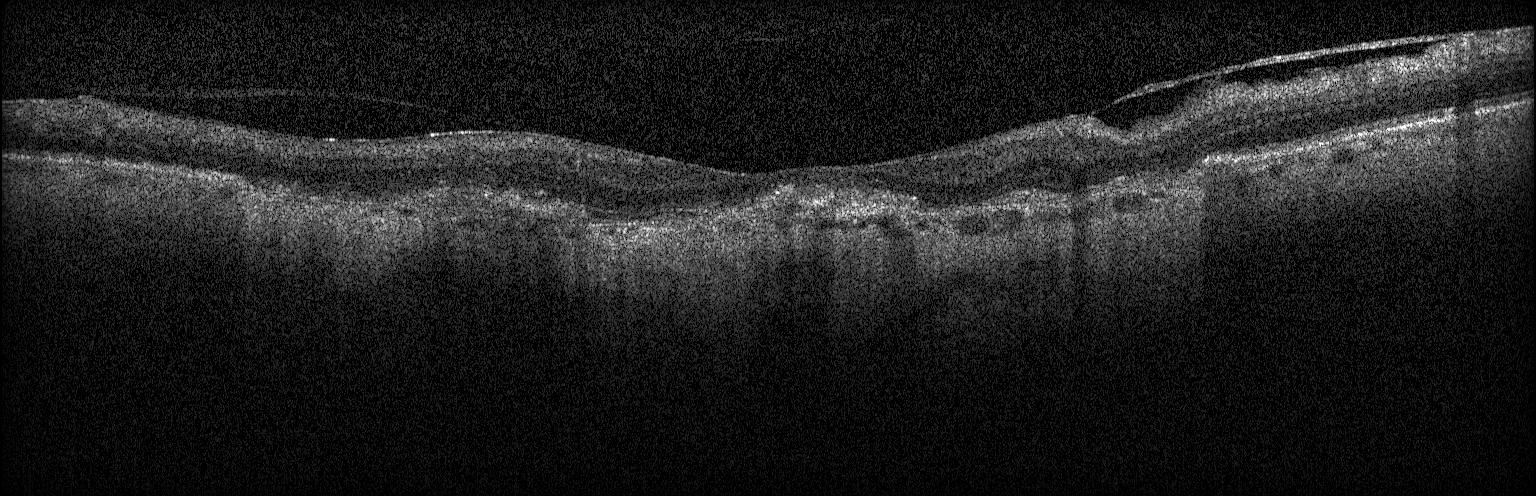
Macular OCT: choroidal neovascularization (CNV).